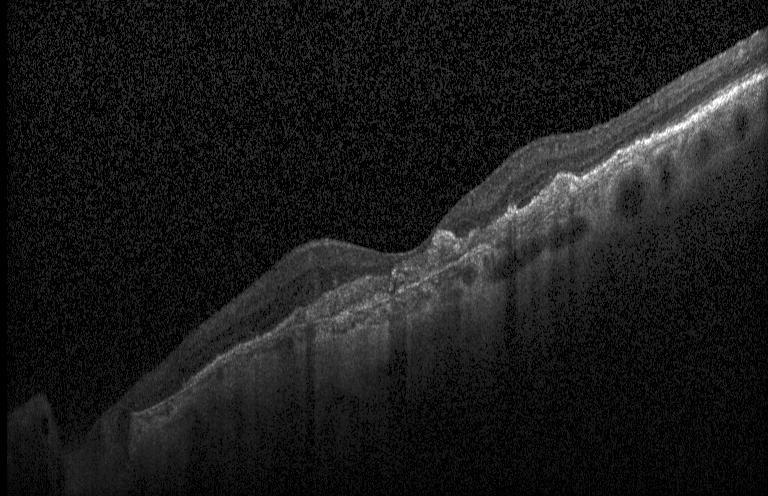

Optical coherence tomography B-scan — This B-scan demonstrates a choroidal neovascular membrane.